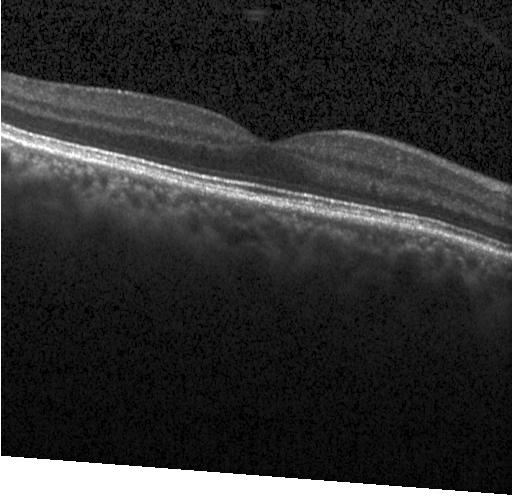
OCT line scan · fovea-centered — The scan shows no CNV, DME, or drusen.